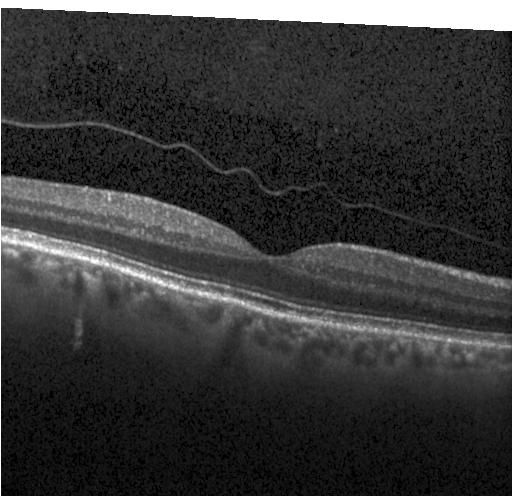
Optical coherence tomography scan · spectral-domain OCT.
Finding: no choroidal neovascularization, diabetic macular edema, or drusen.